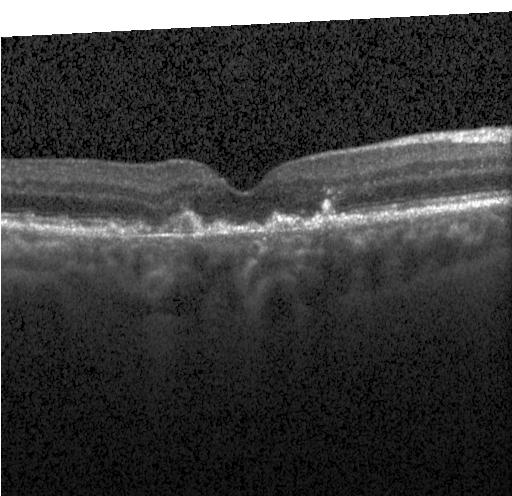
Centered on the fovea. Optical coherence tomography scan
The scan shows choroidal neovascularization.